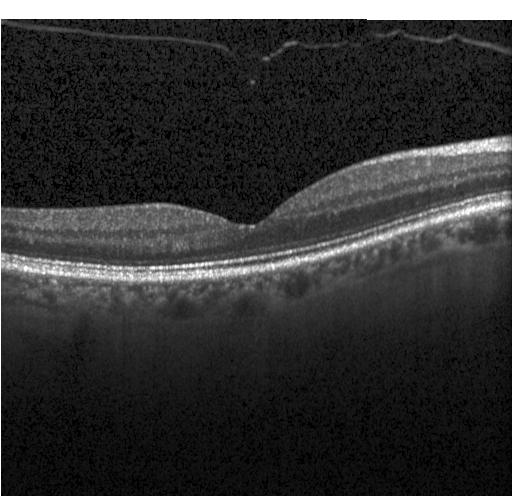 Heidelberg Spectralis OCT system; optical coherence tomography scan. Dx: no evidence of choroidal neovascularization, diabetic macular edema, or drusen.